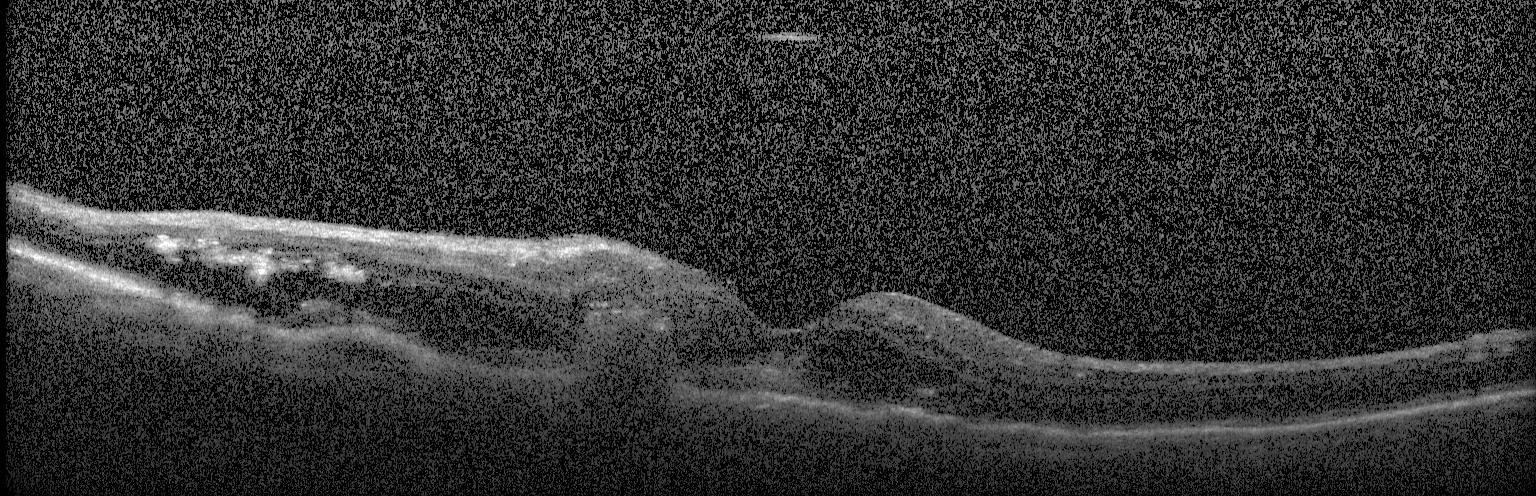

Impression: a choroidal neovascular membrane.